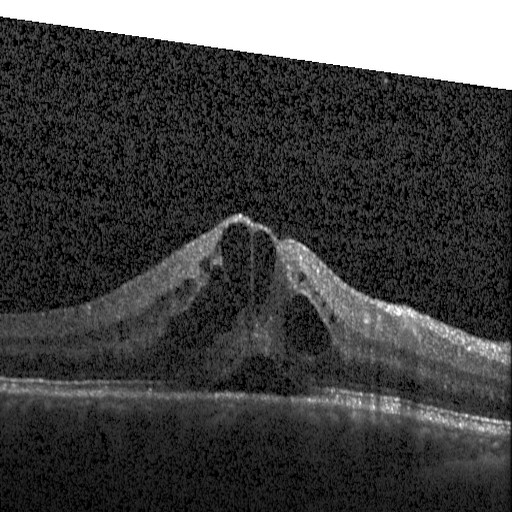
Retinal OCT B-scan
Impression: diabetic macular edema (DME).